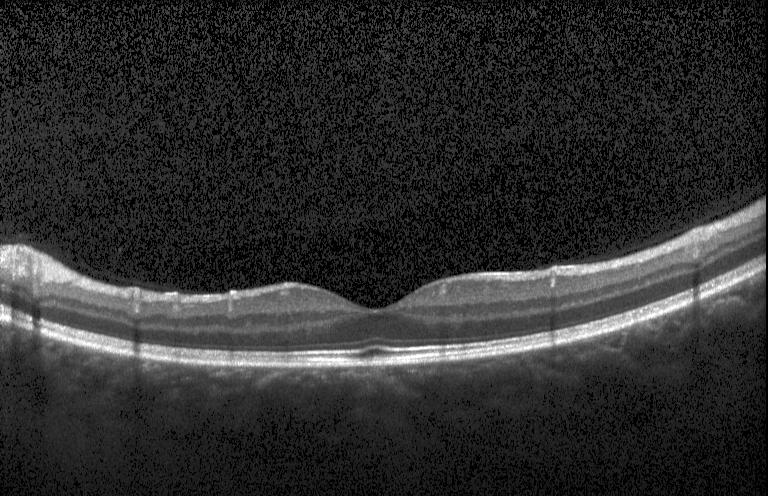

Optical coherence tomography B-scan. SD-OCT.
Finding: neither choroidal neovascularization, diabetic macular edema, nor drusen.